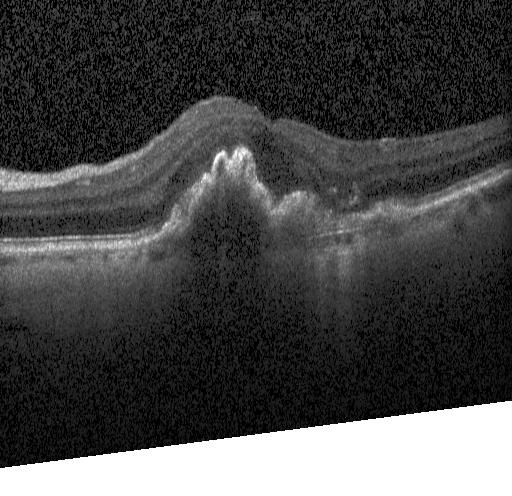

This B-scan demonstrates a choroidal neovascular membrane.